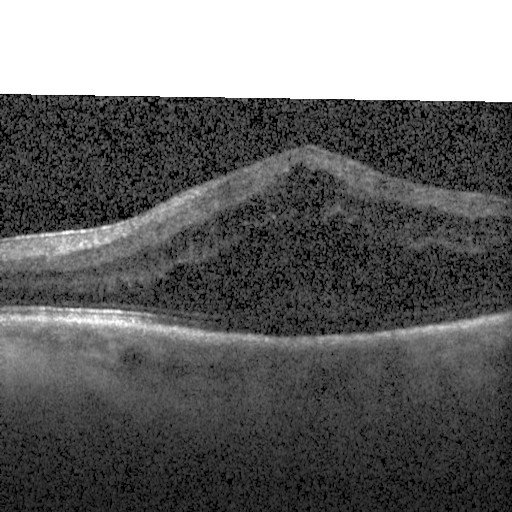

Diagnosis: diabetic macular edema.